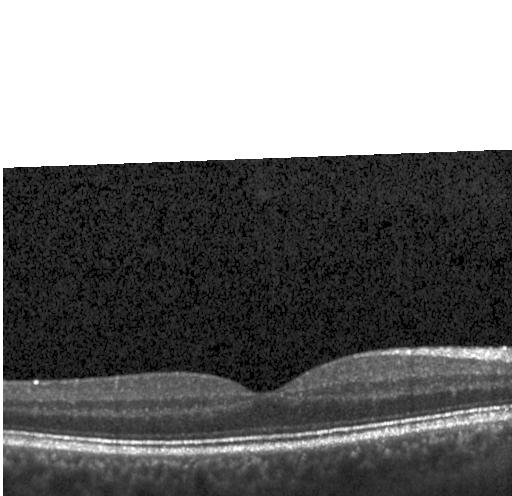 Macular OCT demonstrating no choroidal neovascularization, diabetic macular edema, or drusen.